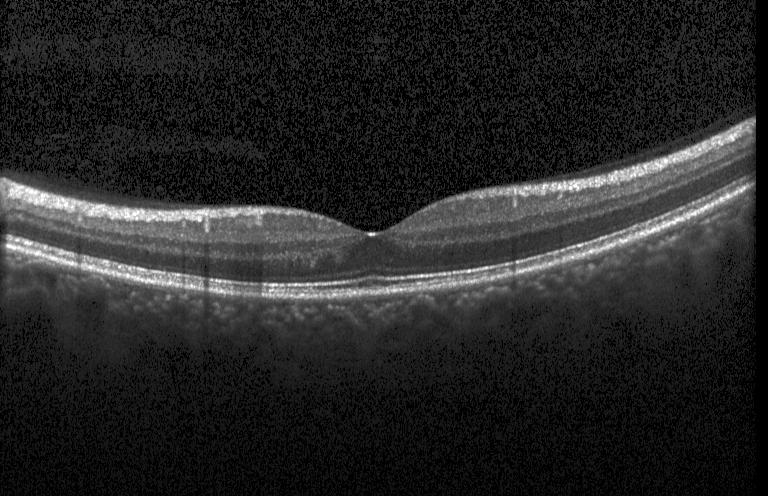 Heidelberg Spectralis · OCT B-scan · horizontal scan through the fovea · spectral-domain OCT. Assessment: no choroidal neovascularization, no diabetic macular edema, and no drusen.